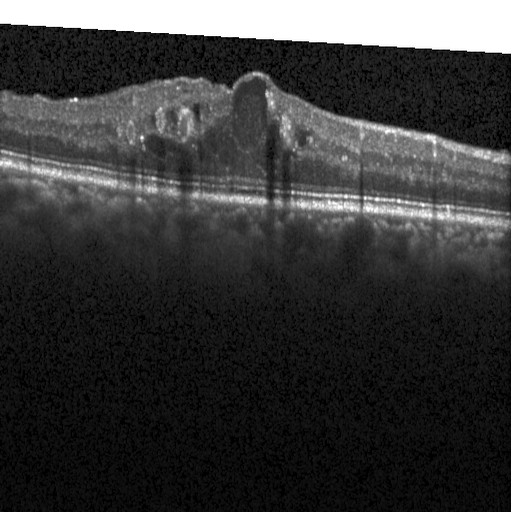 Impression: diabetic macular edema (DME).